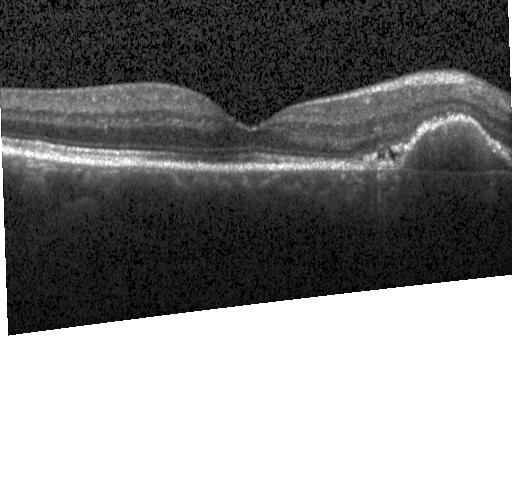
The scan shows CNV.